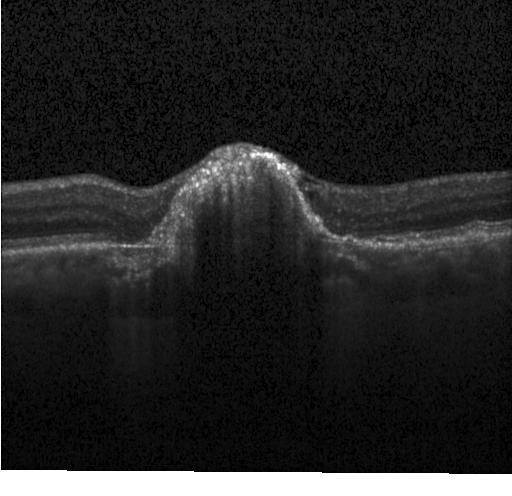
Dx: choroidal neovascularization (CNV).